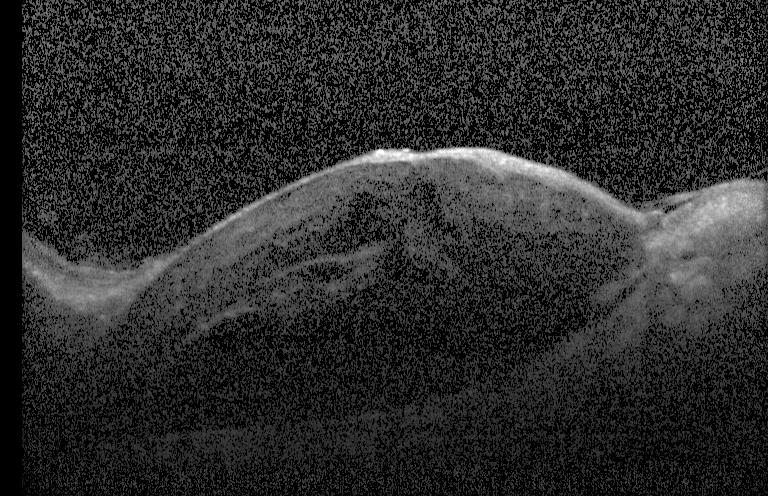

Through the macula; Heidelberg Spectralis OCT system; spectral-domain optical coherence tomography; optical coherence tomography B-scan
Diagnosis: diabetic macular edema (DME).